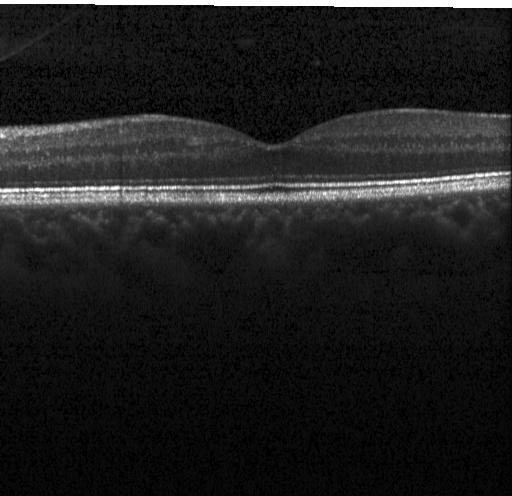 Optical coherence tomography scan.
Finding: neither CNV, DME, nor drusen.